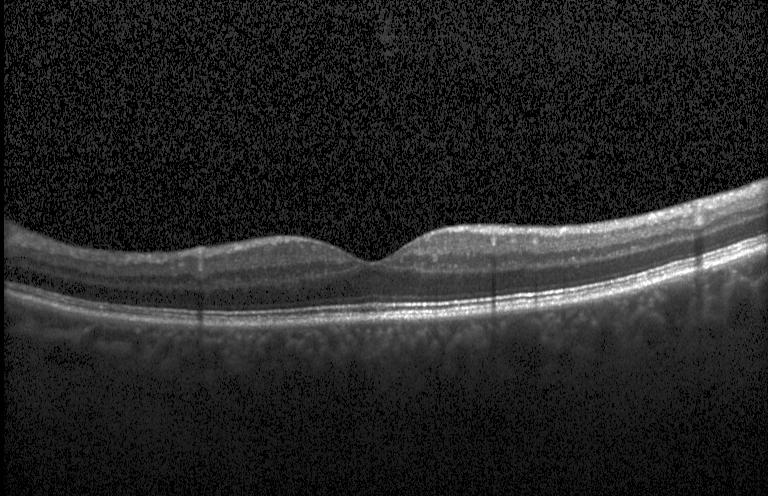

Retinal OCT B-scan.
The scan shows no choroidal neovascularization, no diabetic macular edema, and no drusen.